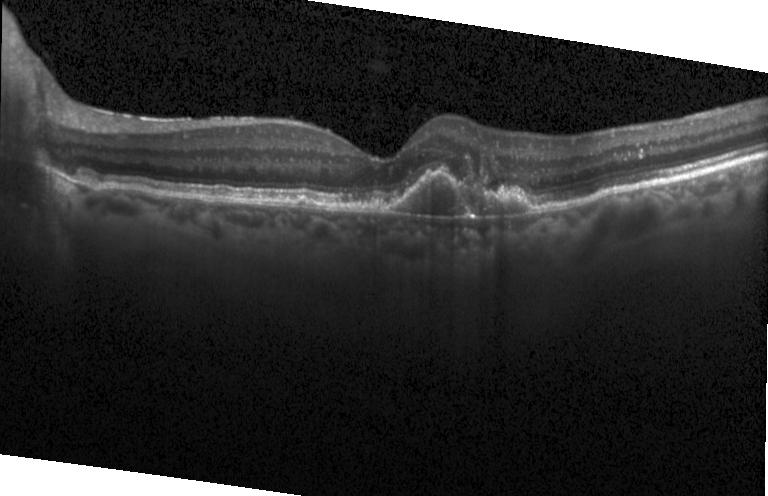
OCT scan showing a choroidal neovascular membrane.